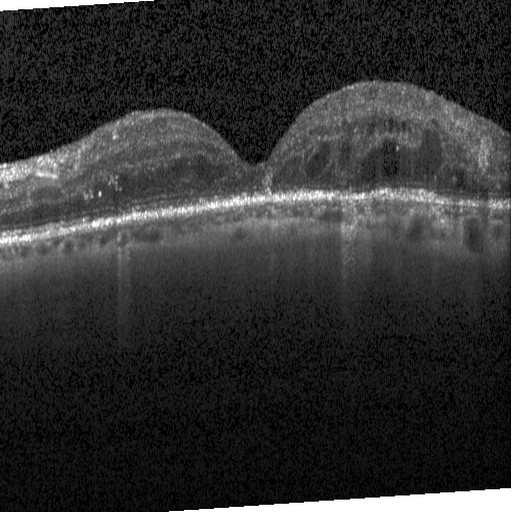
Macular OCT: DME.